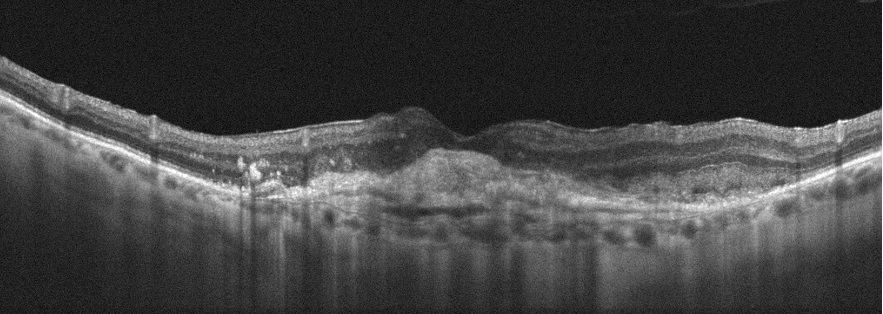
Instrument: Optovue Avanti RTVue XR · fovea-centered · OCT line scan — This B-scan demonstrates age-related macular degeneration (AMD).